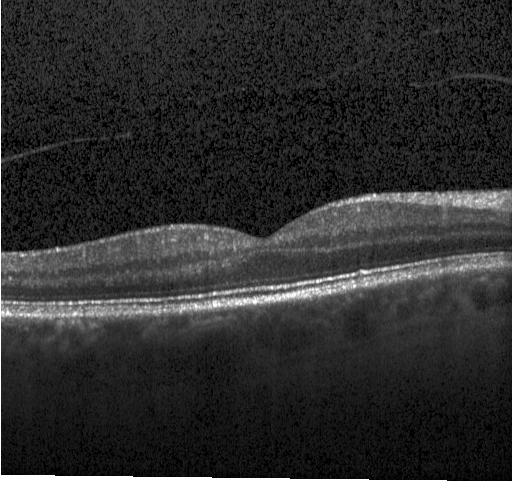
Dx: neither choroidal neovascularization, diabetic macular edema, nor drusen.